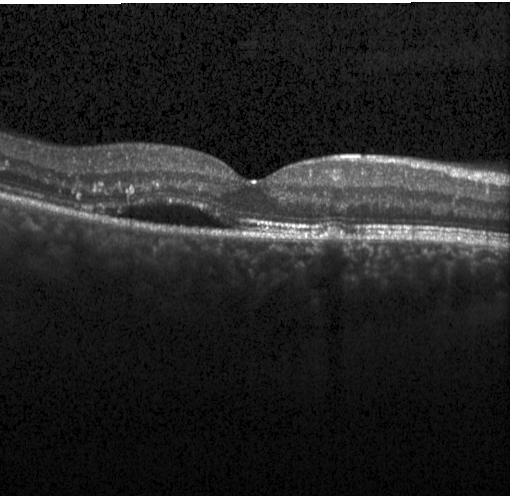

Optical coherence tomography scan, centered on the fovea — Macular OCT: a choroidal neovascular membrane.